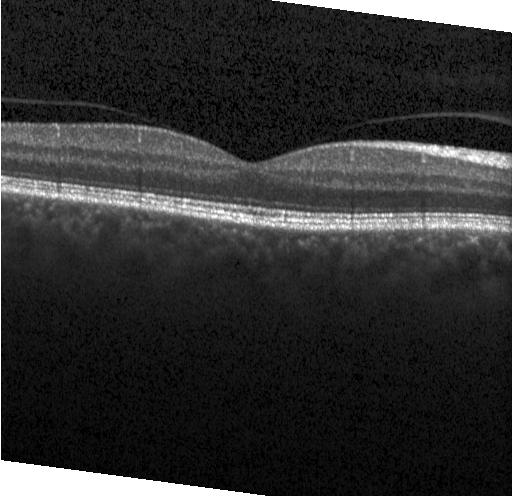 Retinal OCT B-scan, SD-OCT — Assessment: no choroidal neovascularization, no diabetic macular edema, and no drusen.